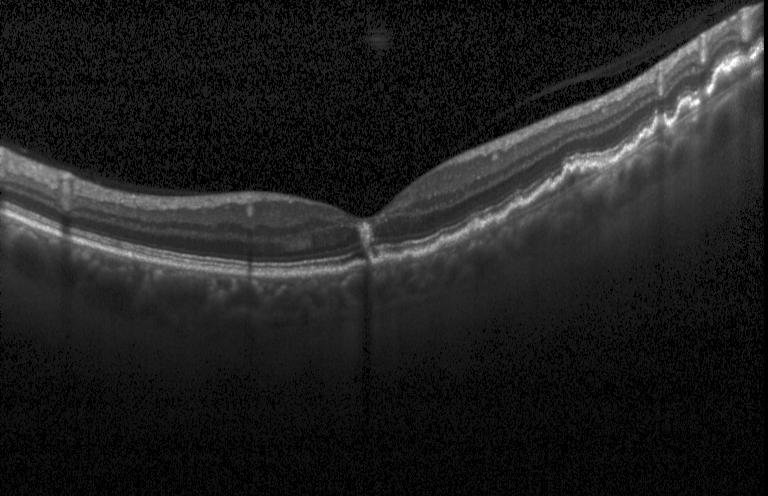 Instrument: Heidelberg Spectralis; spectral-domain optical coherence tomography; through the macula; optical coherence tomography scan
Diagnosis: a choroidal neovascular membrane.